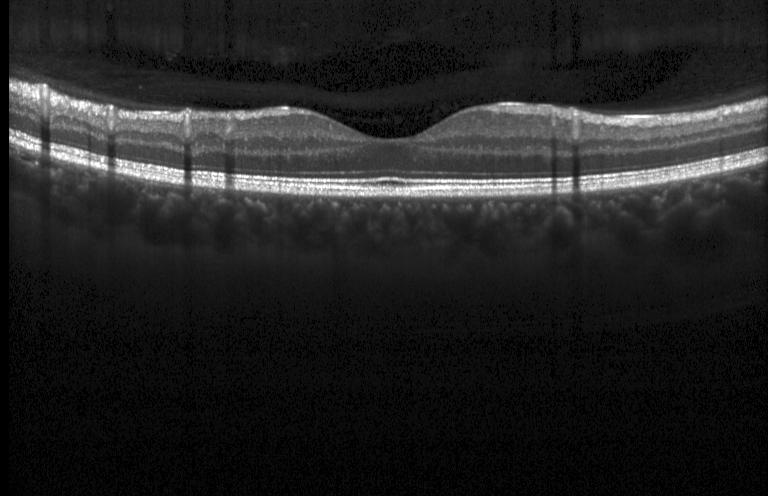
Spectral-domain OCT B-scan: no evidence of CNV, DME, or drusen.